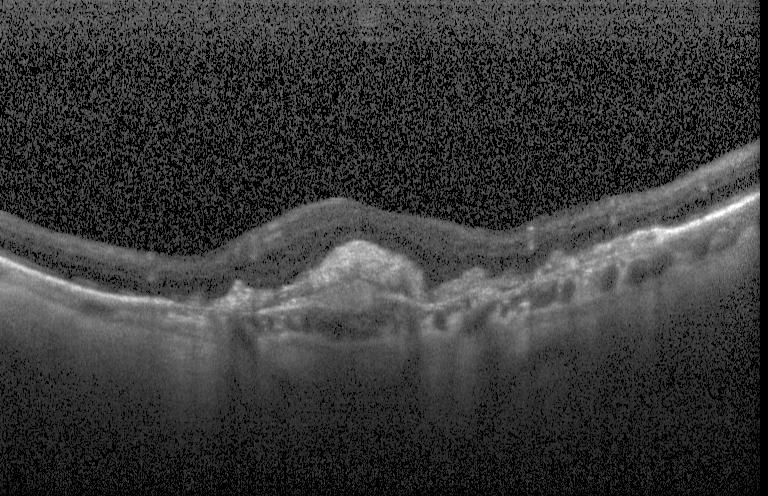

Fovea-centered, Heidelberg Spectralis, OCT line scan, SD-OCT. OCT finding: a choroidal neovascular membrane.